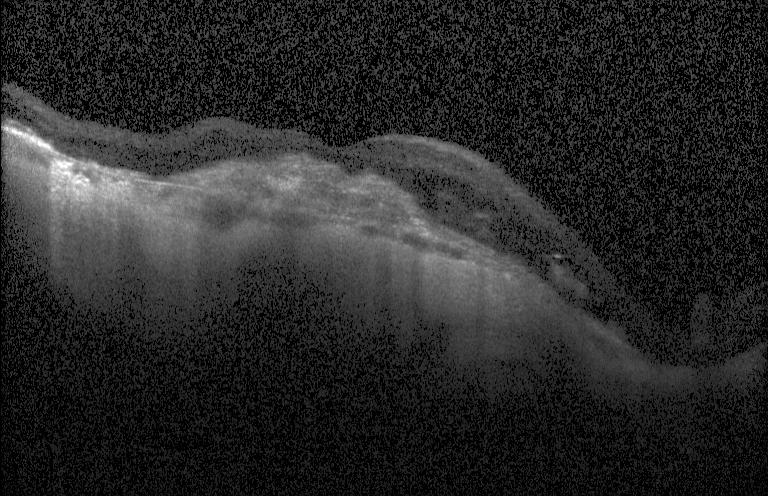
The scan shows choroidal neovascularization.